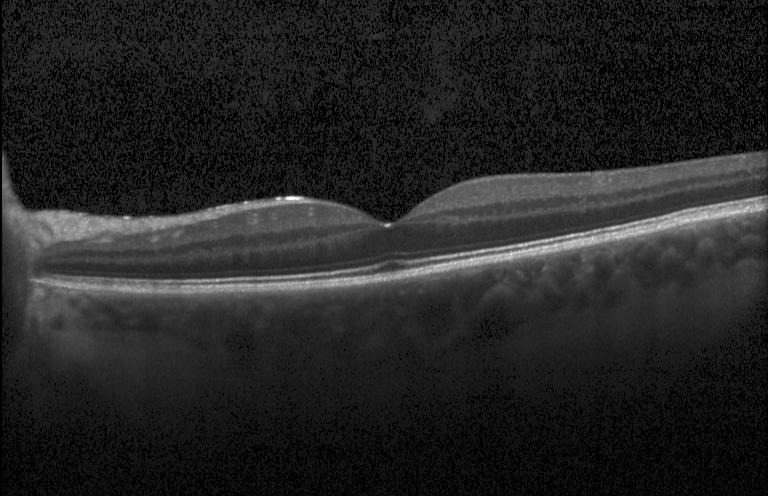

Spectral-domain OCT · OCT line scan · acquired on a Heidelberg Spectralis · macular scan.
OCT finding: no evidence of CNV, DME, or drusen.